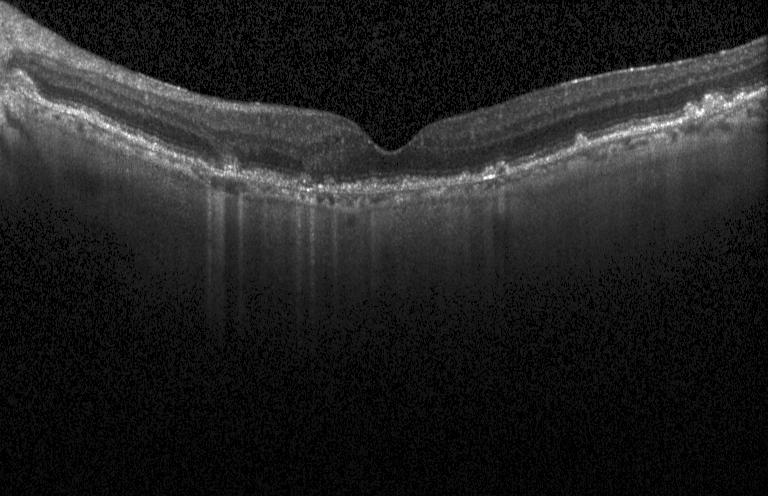 Retinal OCT cross-section · spectral-domain optical coherence tomography — Impression: choroidal neovascularization (CNV).